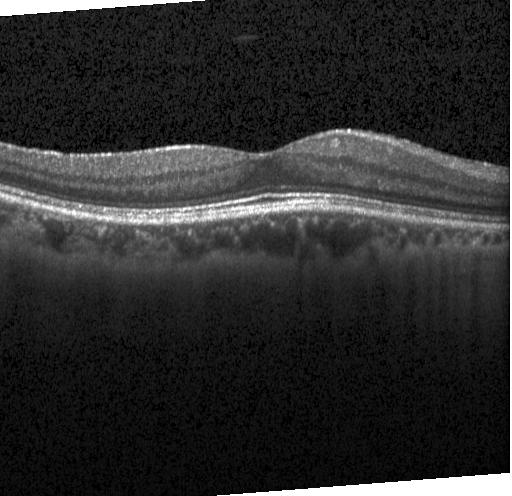
Finding: no choroidal neovascularization, no diabetic macular edema, and no drusen.